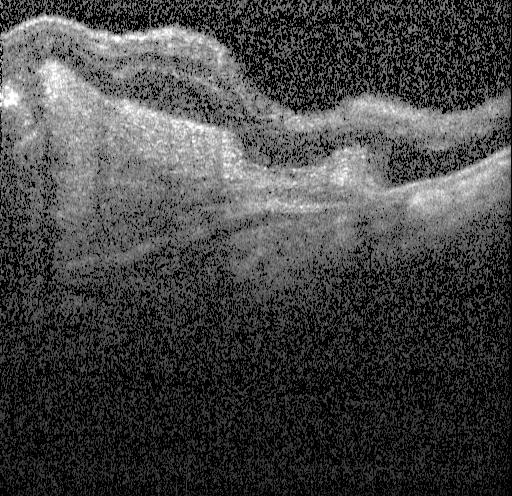
Finding: choroidal neovascularization (CNV).